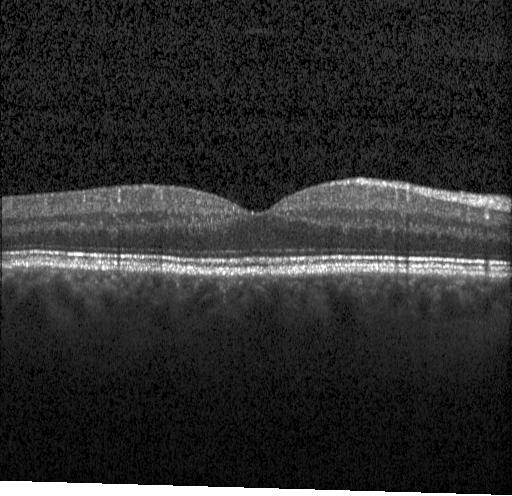 Macular OCT: no CNV, no DME, and no drusen.